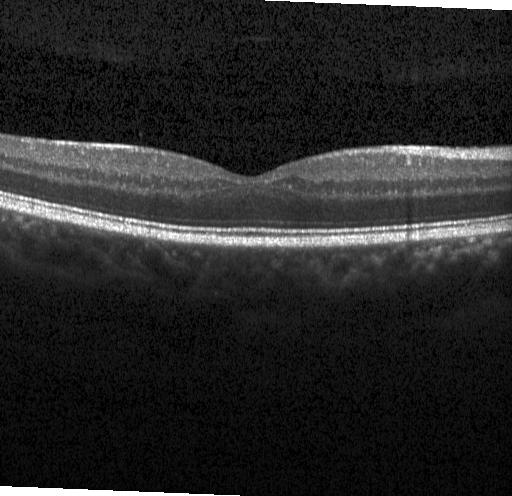
Through the macula, optical coherence tomography B-scan, instrument: Heidelberg Spectralis.
Diagnosis: no evidence of choroidal neovascularization, diabetic macular edema, or drusen.